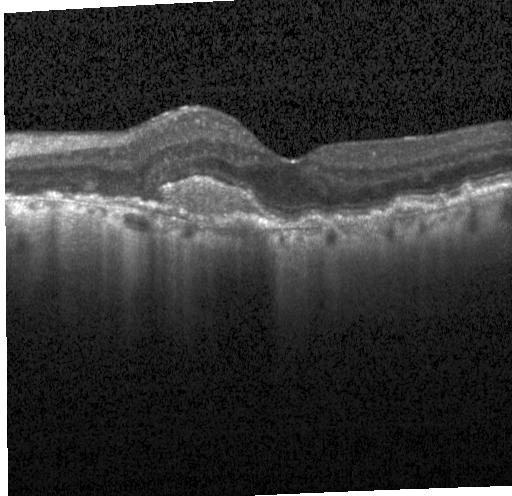 Impression: CNV.